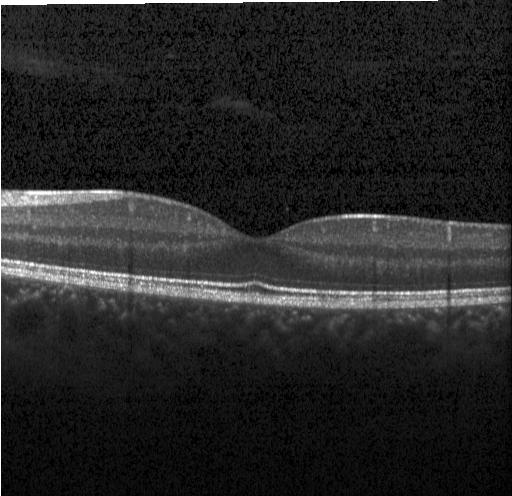 Retinal OCT cross-section. Through the macula
This B-scan demonstrates no evidence of choroidal neovascularization, diabetic macular edema, or drusen.